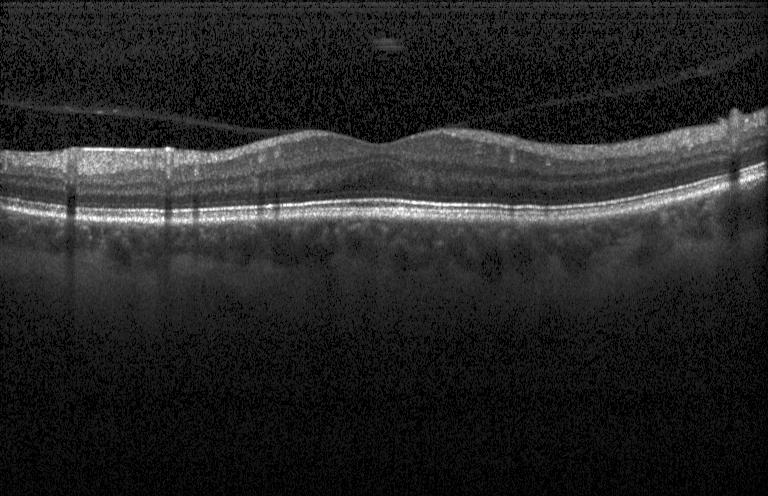

Spectral-domain OCT B-scan: neither choroidal neovascularization, diabetic macular edema, nor drusen.